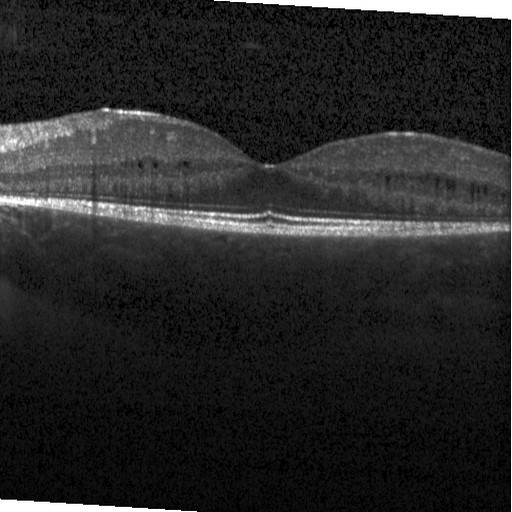 This B-scan demonstrates DME.